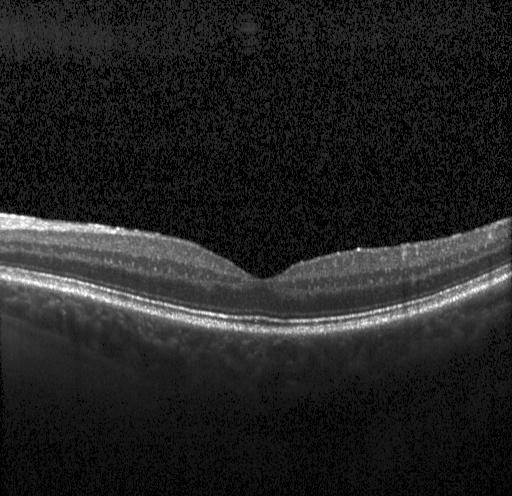 Horizontal scan through the fovea, retinal OCT cross-section — The scan shows no choroidal neovascularization, diabetic macular edema, or drusen.